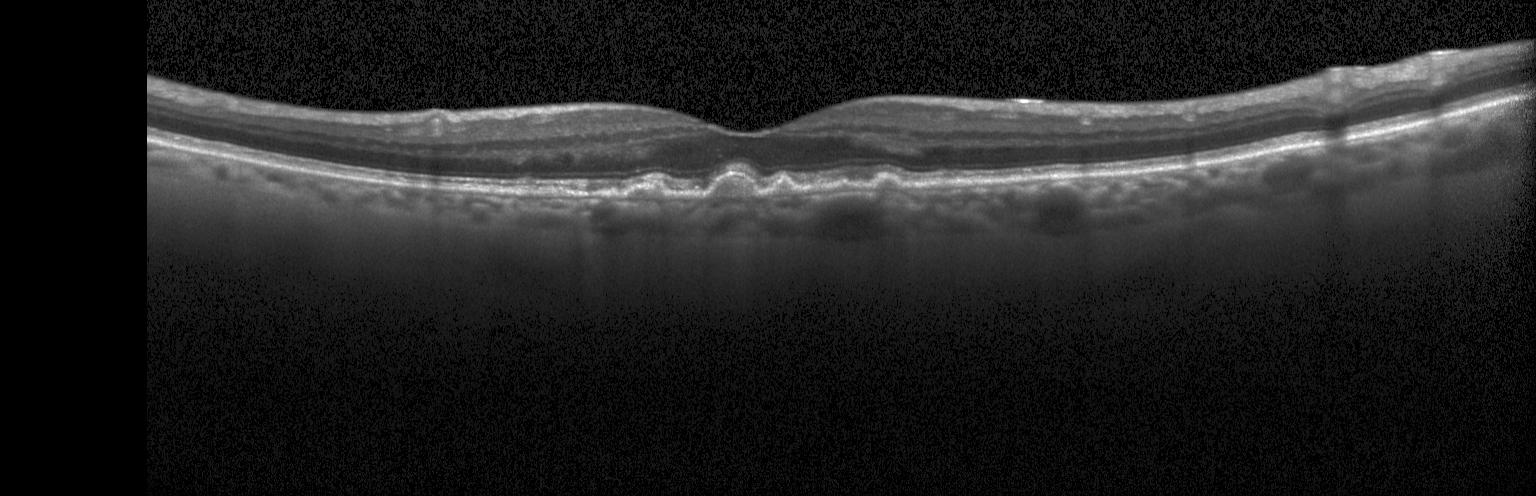

Fovea-centered. Spectral-domain OCT. OCT B-scan. Acquired on a Heidelberg Spectralis
Finding: sub-RPE drusenoid deposits.